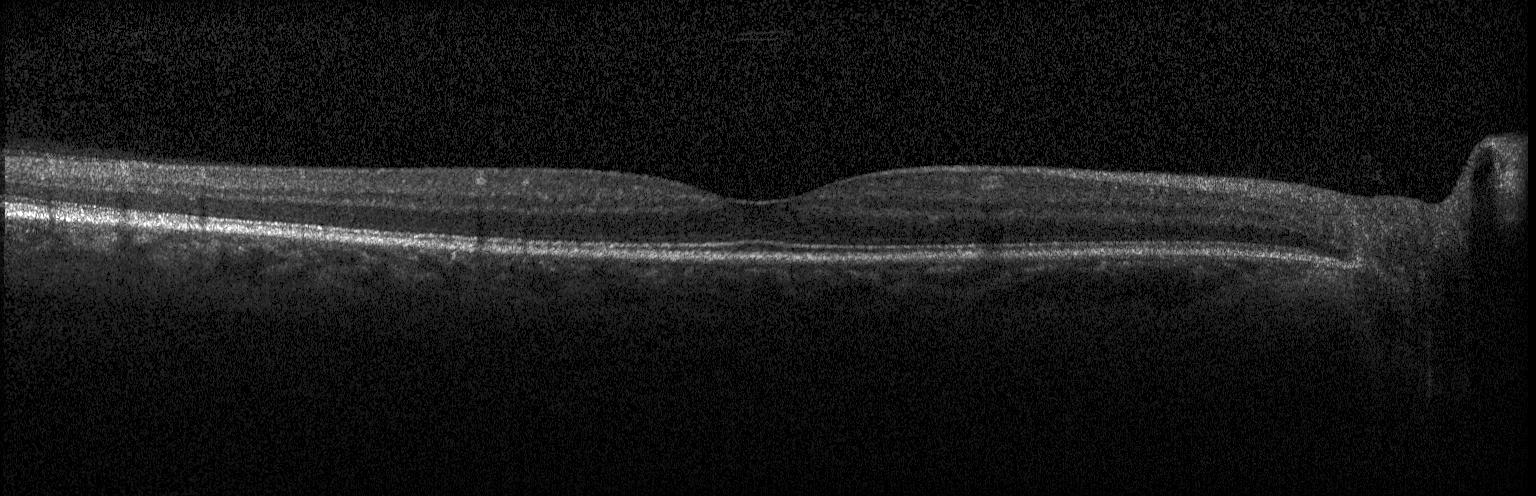 Heidelberg Spectralis OCT system · spectral-domain OCT · OCT B-scan · horizontal scan through the fovea. No evidence of CNV, DME, or drusen.